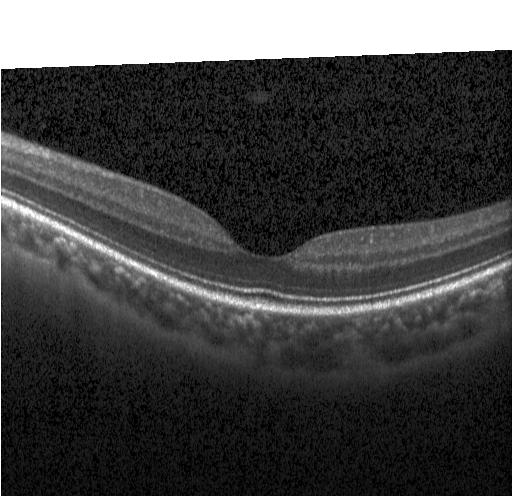 SD-OCT, macular scan, optical coherence tomography scan
OCT finding: no choroidal neovascularization, no diabetic macular edema, and no drusen.